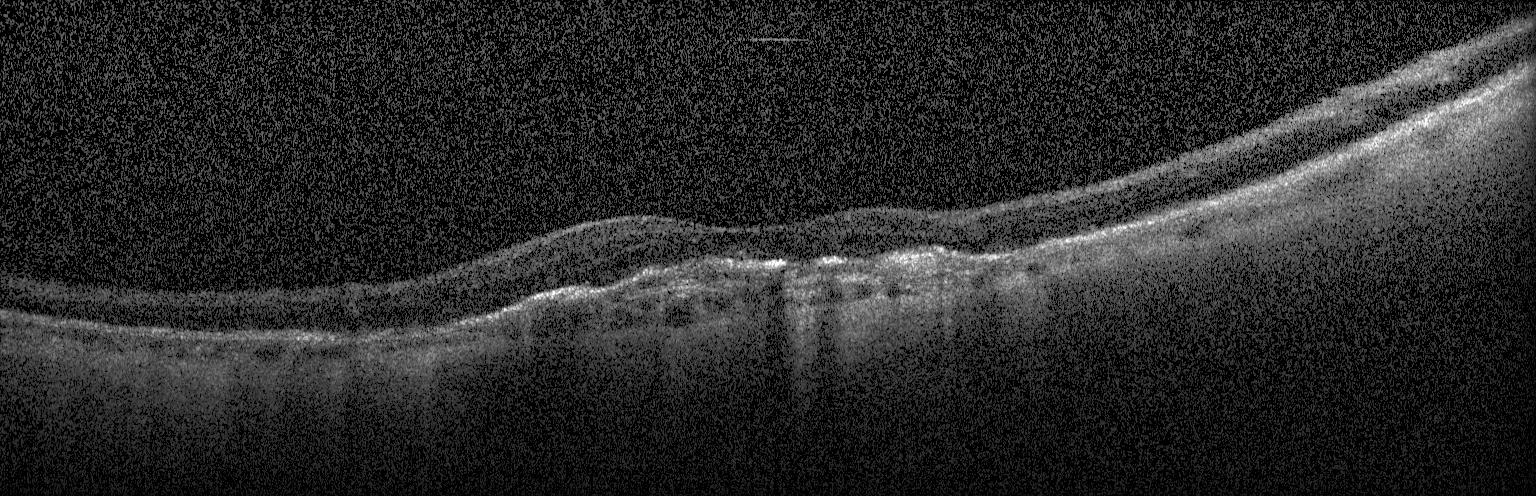
Macular OCT: a choroidal neovascular membrane.